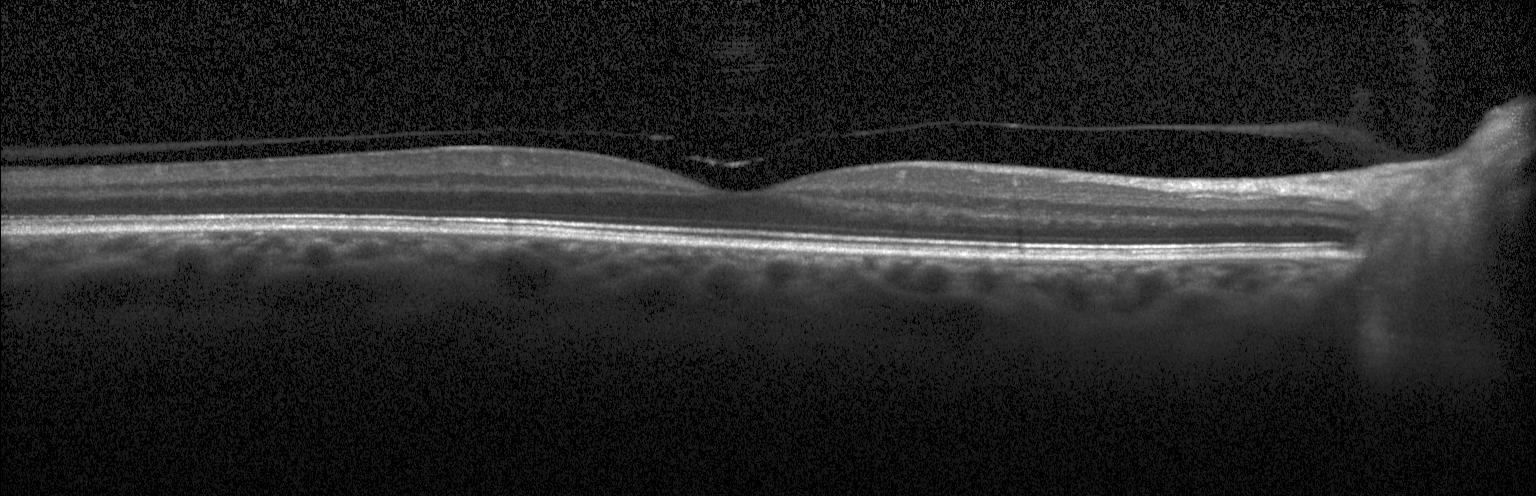
Optical coherence tomography scan. Dx: no choroidal neovascularization, no diabetic macular edema, and no drusen.